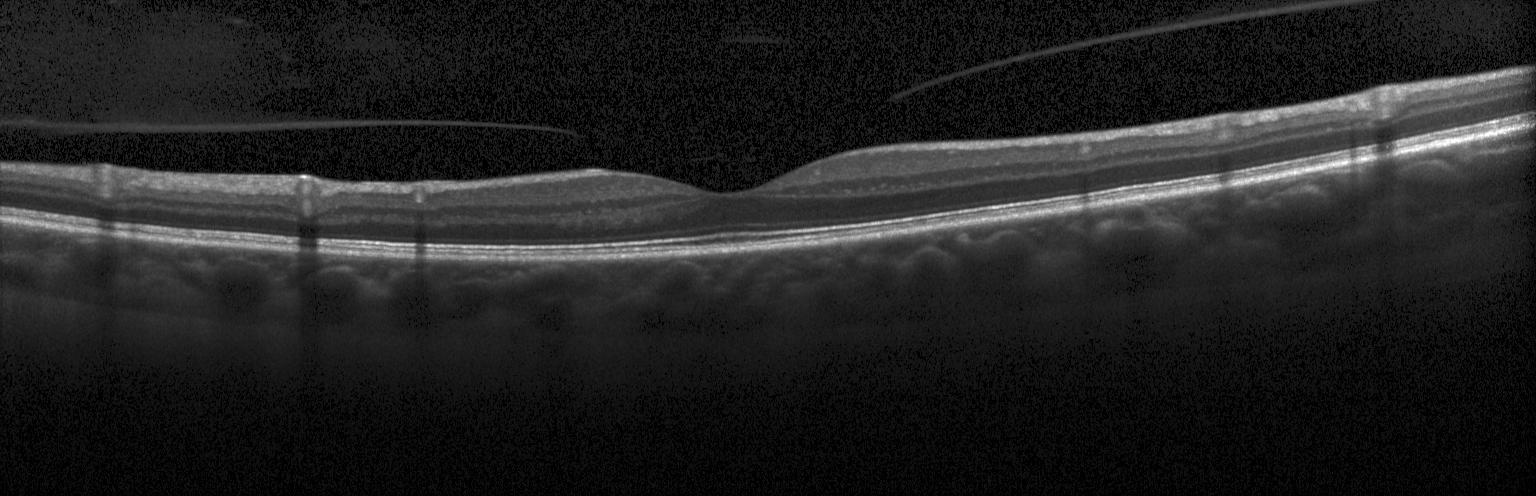

Fovea-centered, retinal OCT B-scan, instrument: Heidelberg Spectralis — Assessment: no choroidal neovascularization, no diabetic macular edema, and no drusen.